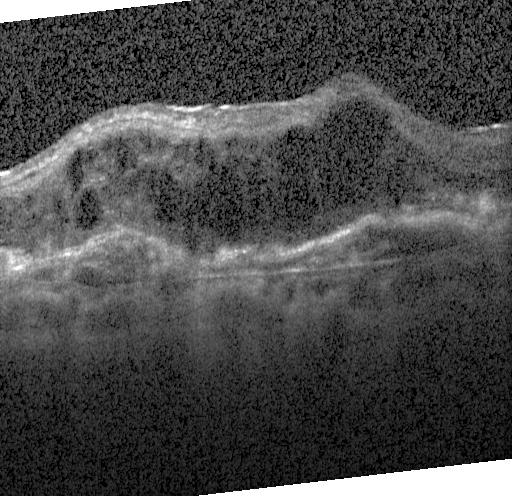

Retinal OCT cross-section · macular scan. Impression: a choroidal neovascular membrane.